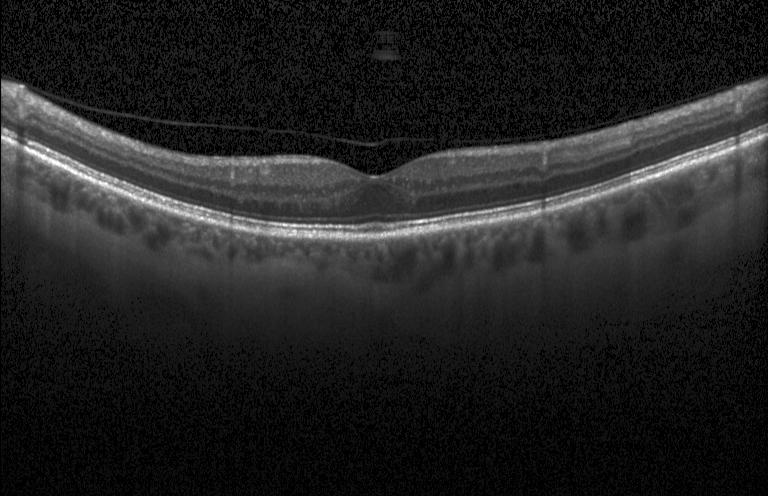
OCT line scan
Finding: no evidence of CNV, DME, or drusen.